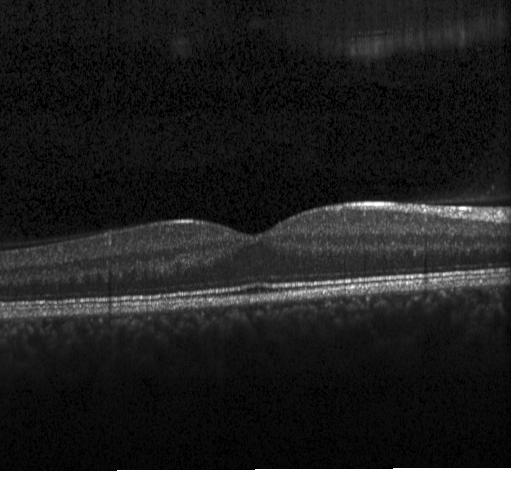
This B-scan demonstrates no choroidal neovascularization, diabetic macular edema, or drusen.